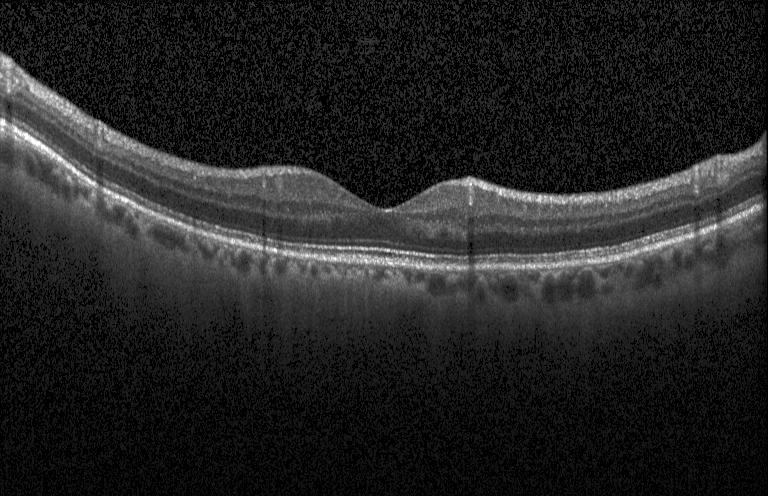 Centered on the fovea, Heidelberg Spectralis OCT system, retinal OCT B-scan, SD-OCT.
Diagnosis: no evidence of CNV, DME, or drusen.